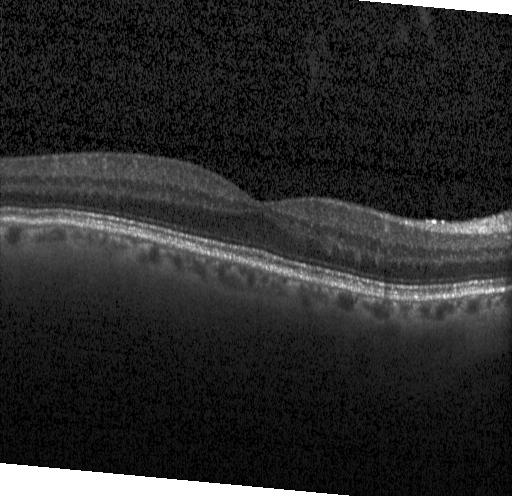 OCT line scan. Instrument: Heidelberg Spectralis. Horizontal scan through the fovea.
Finding: no choroidal neovascularization, no diabetic macular edema, and no drusen.